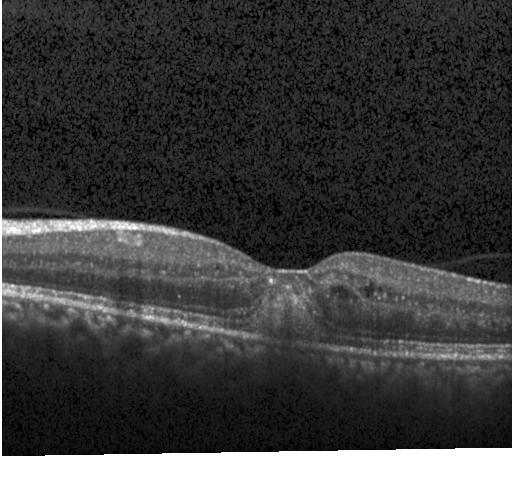

Acquired on a Heidelberg Spectralis · optical coherence tomography B-scan. CNV.